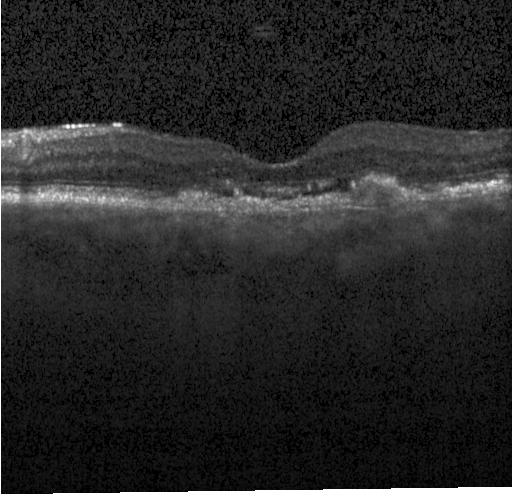 Optical coherence tomography scan · acquired on a Heidelberg Spectralis.
A choroidal neovascular membrane.